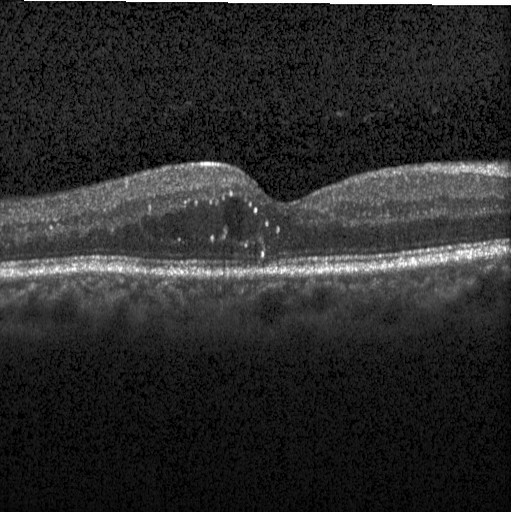
OCT B-scan; Heidelberg Spectralis OCT system; horizontal scan through the fovea; spectral-domain OCT.
Impression: diabetic macular edema.